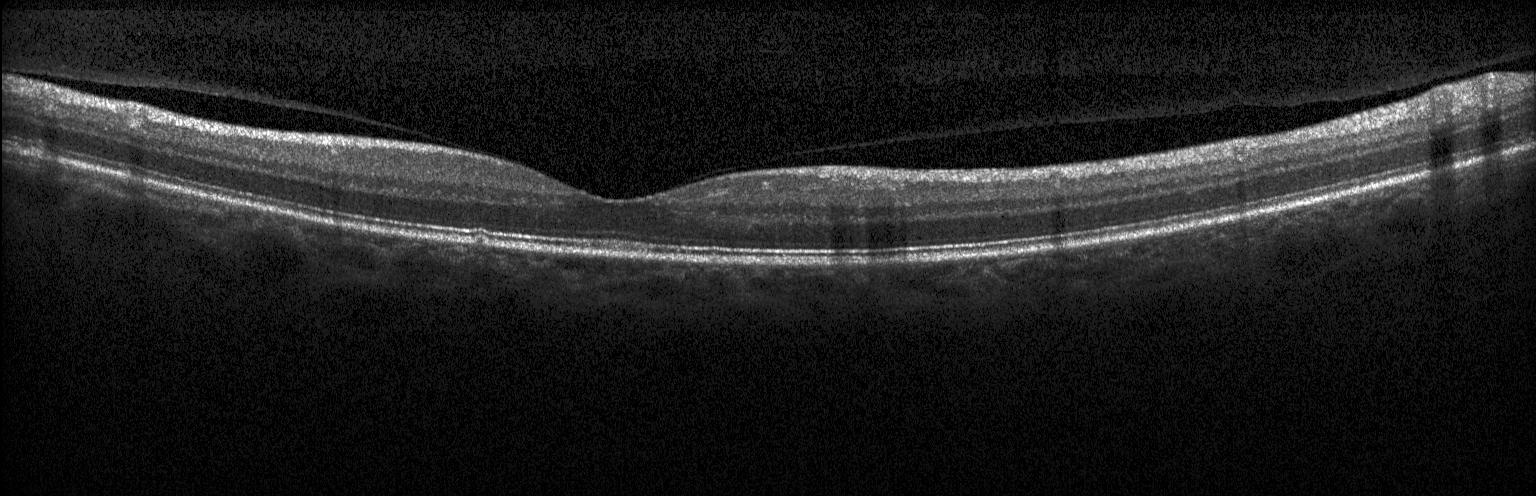 Retinal OCT B-scan. Impression: no choroidal neovascularization, diabetic macular edema, or drusen.